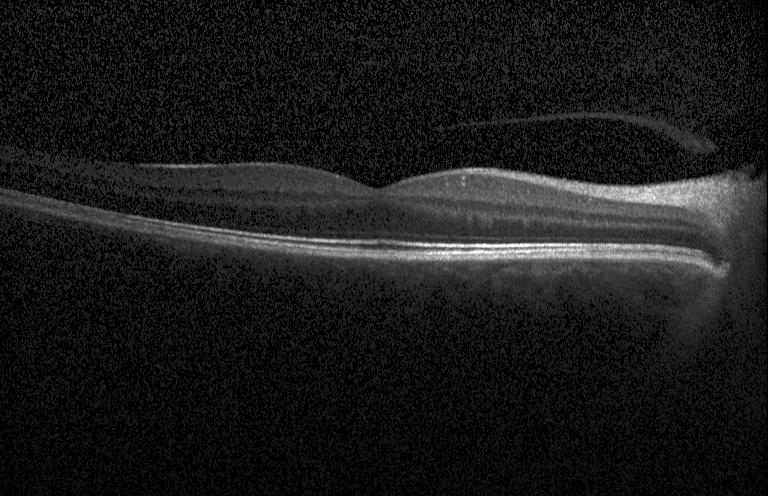
Optical coherence tomography B-scan, spectral-domain optical coherence tomography.
Finding: no evidence of choroidal neovascularization, diabetic macular edema, or drusen.